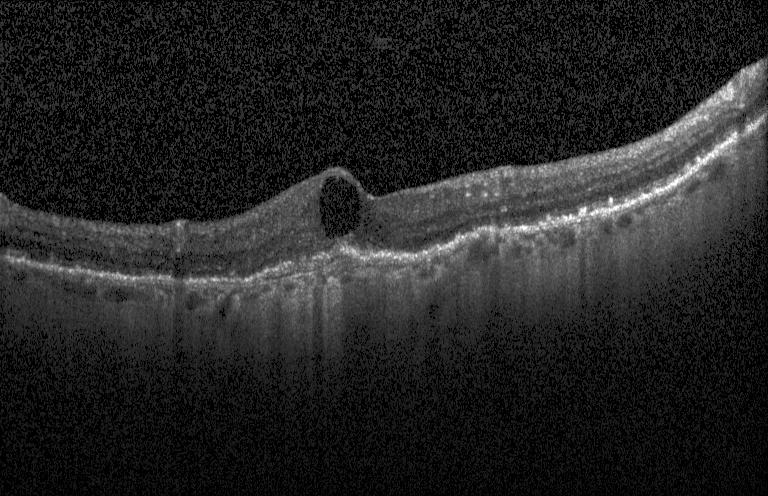
Optical coherence tomography B-scan.
OCT finding: a choroidal neovascular membrane.